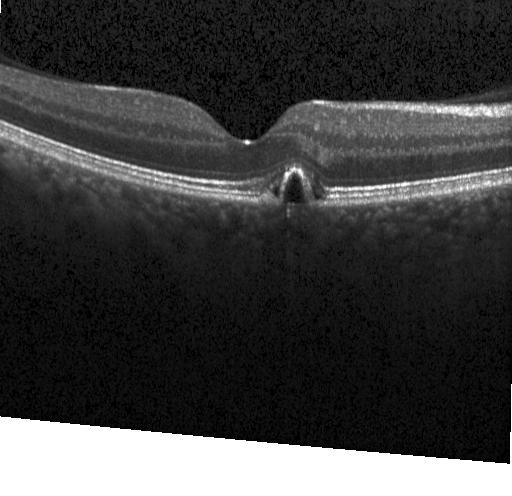
Finding: a choroidal neovascular membrane.